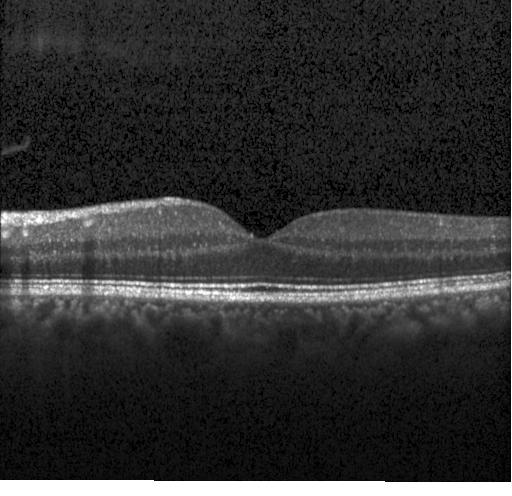

Assessment: no CNV, DME, or drusen.